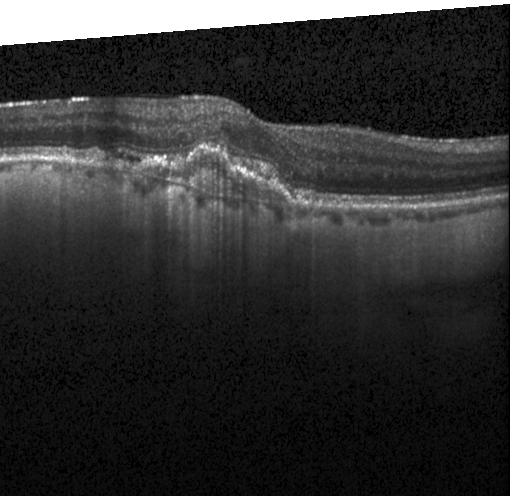
Impression: CNV.